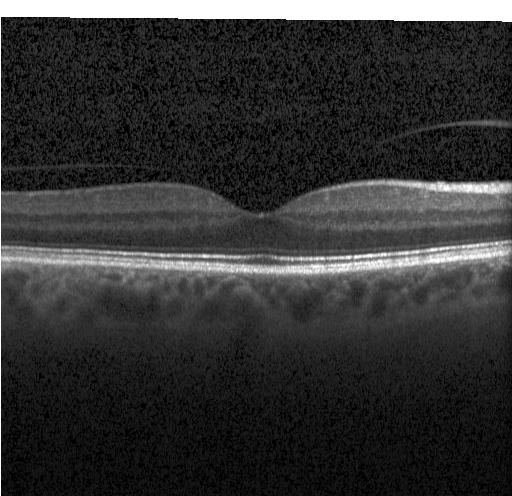 Heidelberg Spectralis. Spectral-domain OCT. Optical coherence tomography B-scan. Horizontal scan through the fovea.
OCT finding: no evidence of choroidal neovascularization, diabetic macular edema, or drusen.